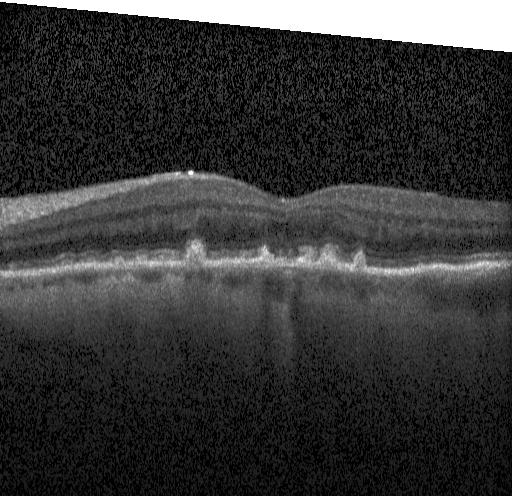

Macular scan · SD-OCT · Heidelberg Spectralis OCT system · retinal OCT cross-section
Diagnosis: multiple drusen.